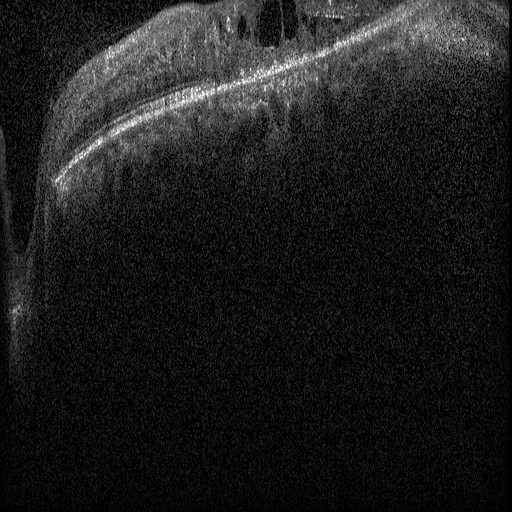
SD-OCT; OCT B-scan. The scan shows DME.